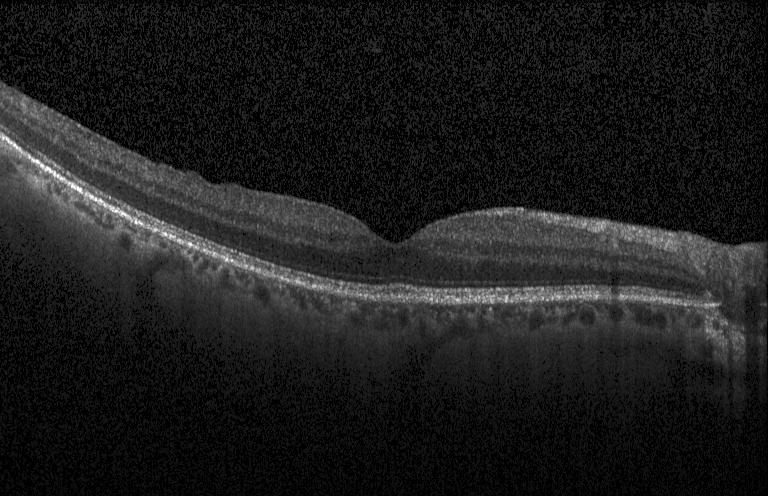

Retinal OCT B-scan · horizontal scan through the fovea. This B-scan demonstrates neither choroidal neovascularization, diabetic macular edema, nor drusen.